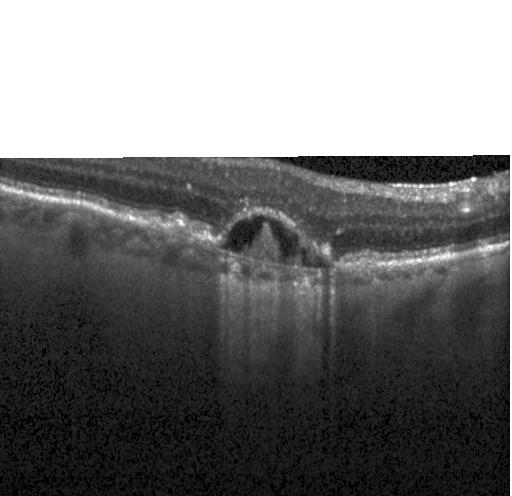

Dx: choroidal neovascularization (CNV).